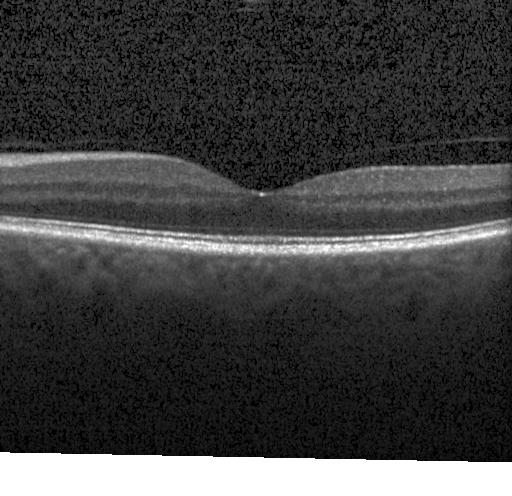 Diagnosis: neither CNV, DME, nor drusen.